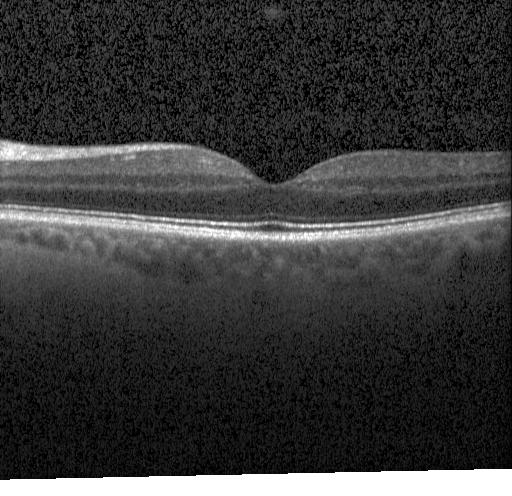

OCT line scan. Diagnosis: neither choroidal neovascularization, diabetic macular edema, nor drusen.